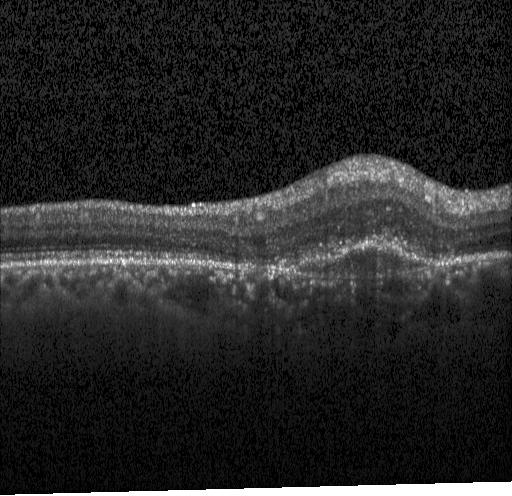

Heidelberg Spectralis, spectral-domain optical coherence tomography, retinal OCT cross-section, macular scan.
Assessment: a choroidal neovascular membrane.